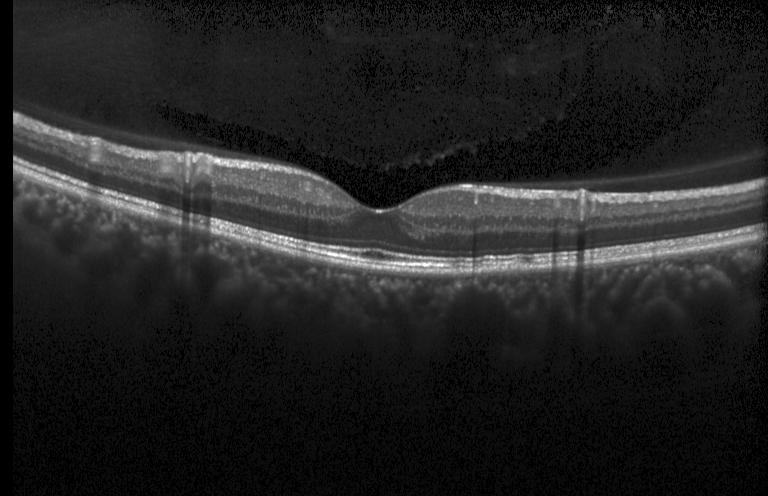 Heidelberg Spectralis. Fovea-centered. Retinal OCT B-scan. SD-OCT.
The scan shows no evidence of choroidal neovascularization, diabetic macular edema, or drusen.